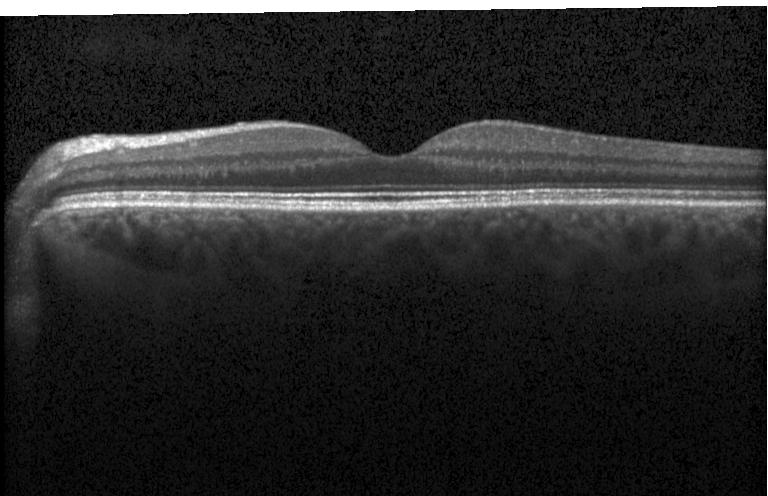 This B-scan demonstrates no choroidal neovascularization, no diabetic macular edema, and no drusen.